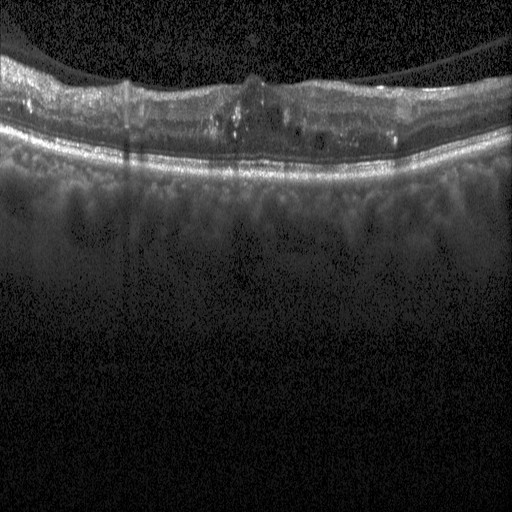

This B-scan demonstrates diabetic macular edema.